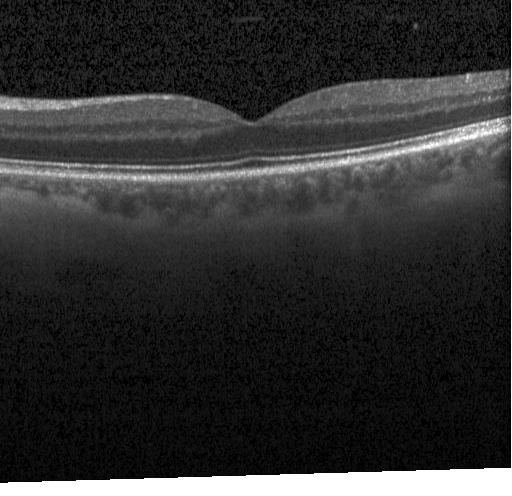
Spectral-domain OCT, Heidelberg Spectralis, macular scan, retinal OCT B-scan.
Finding: no evidence of choroidal neovascularization, diabetic macular edema, or drusen.